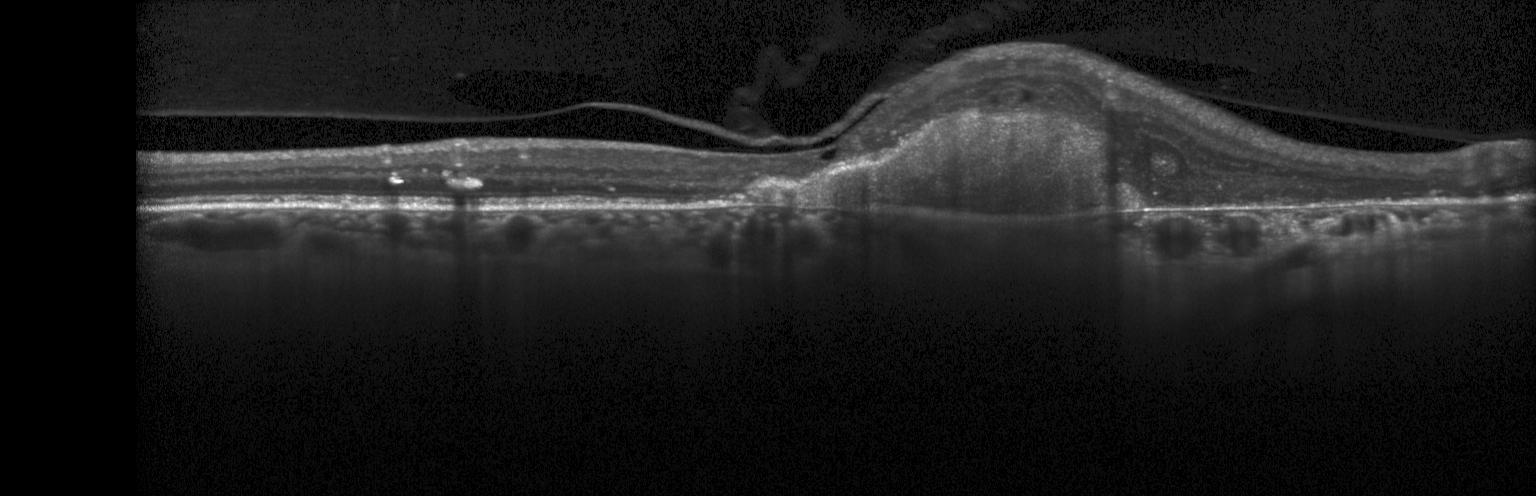

OCT B-scan. OCT finding: a choroidal neovascular membrane.